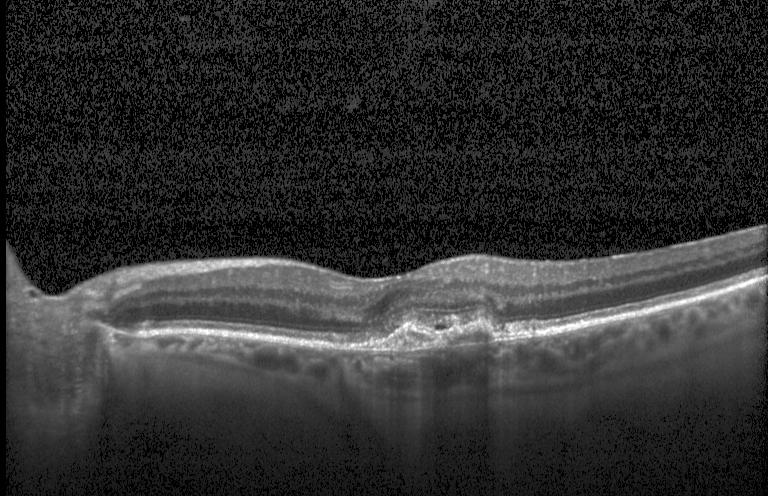

This B-scan demonstrates choroidal neovascularization.